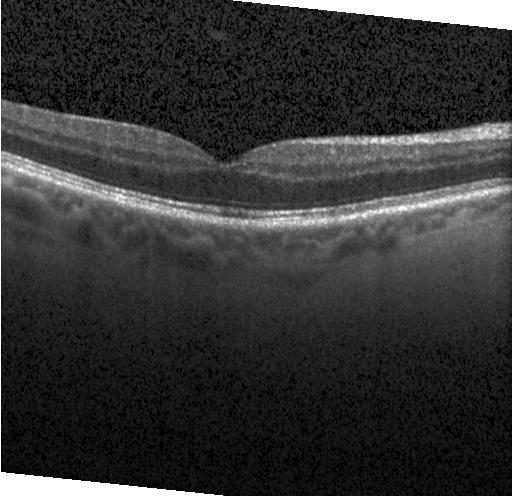 Retinal OCT B-scan.
The scan shows no evidence of choroidal neovascularization, diabetic macular edema, or drusen.